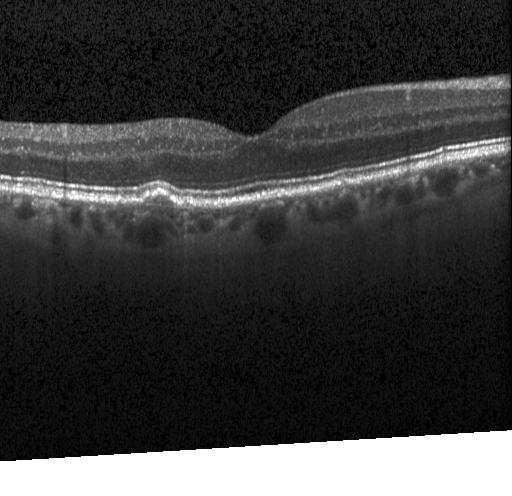
OCT B-scan showing multiple drusen.